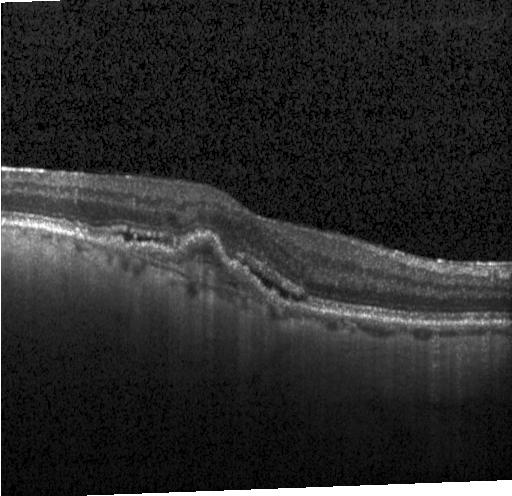
Diagnosis: CNV.